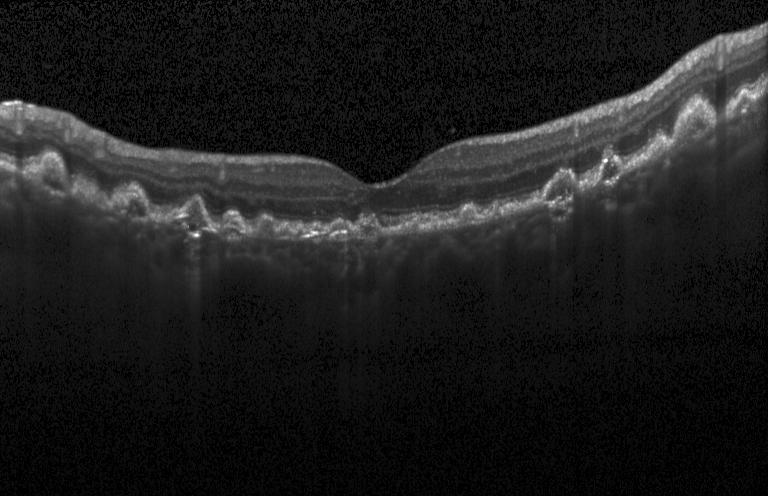

Retinal OCT B-scan
This B-scan demonstrates CNV.